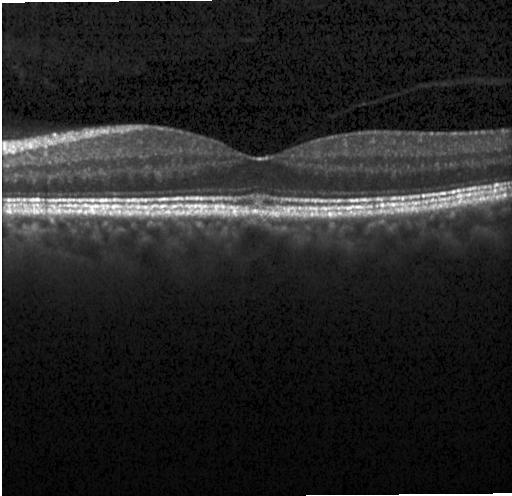

OCT B-scan. Dx: no choroidal neovascularization, diabetic macular edema, or drusen.